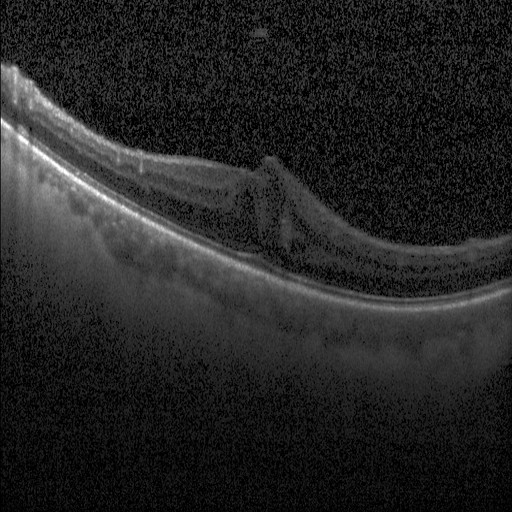
The scan shows diabetic macular edema (DME).